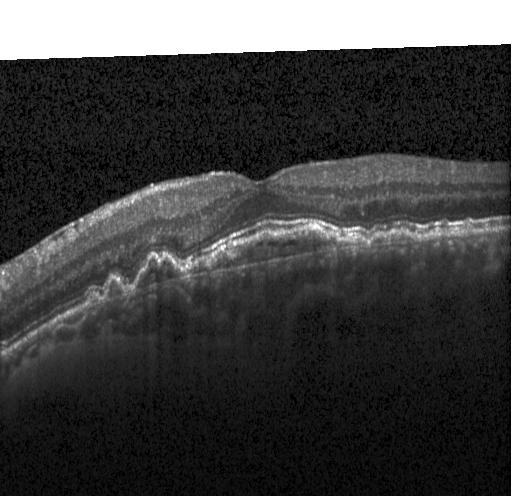

Macular scan · optical coherence tomography B-scan
Finding: a choroidal neovascular membrane.